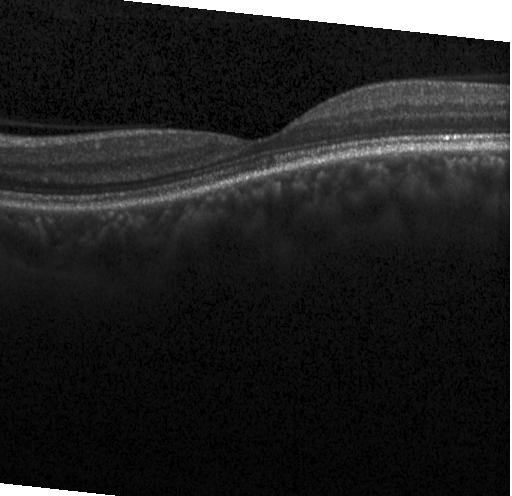 Fovea-centered · spectral-domain OCT · OCT line scan.
The scan shows neither choroidal neovascularization, diabetic macular edema, nor drusen.